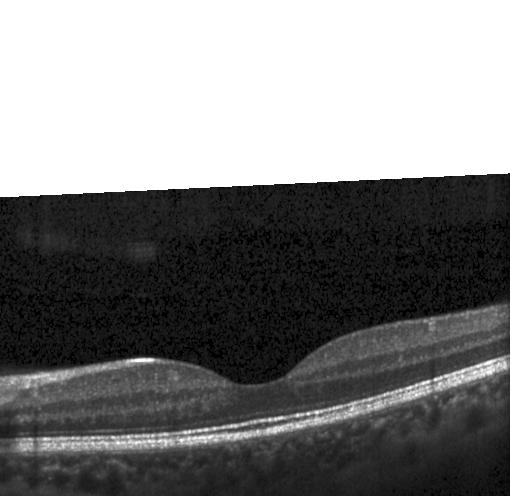
Macular OCT: neither choroidal neovascularization, diabetic macular edema, nor drusen.